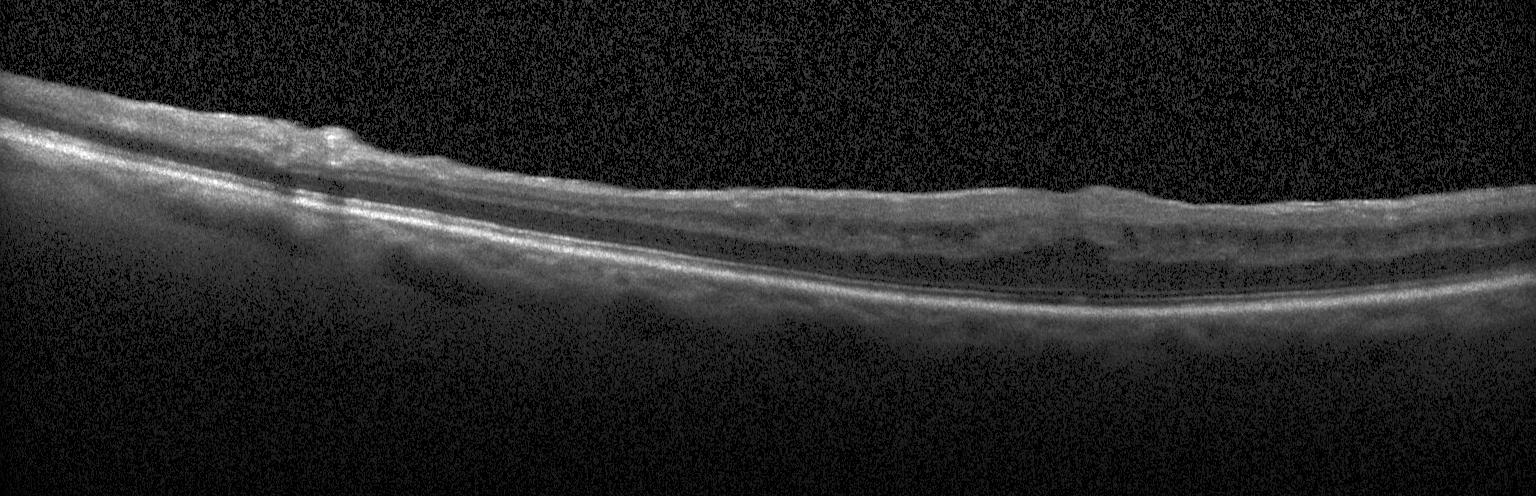
OCT B-scan showing DME.